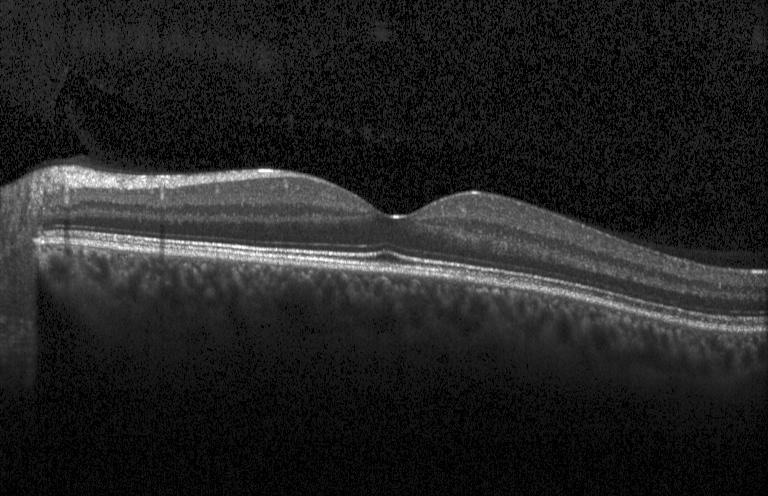
Finding: no choroidal neovascularization, no diabetic macular edema, and no drusen.